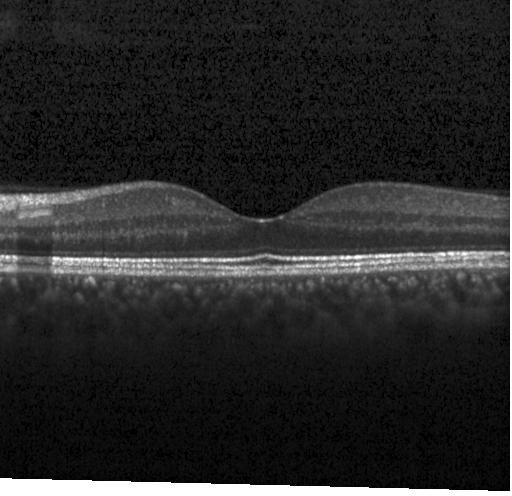 OCT finding: neither choroidal neovascularization, diabetic macular edema, nor drusen.